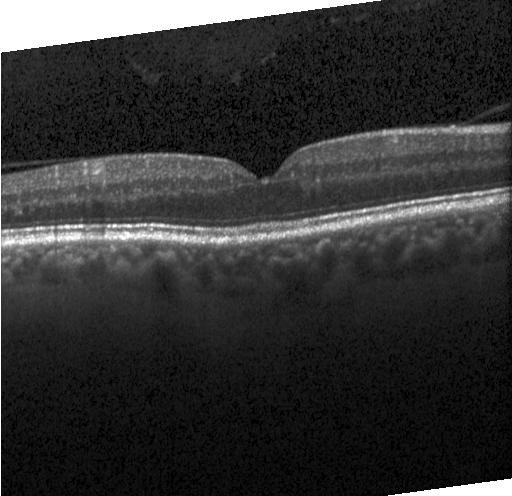

Optical coherence tomography scan, spectral-domain optical coherence tomography. Macular OCT: no choroidal neovascularization, diabetic macular edema, or drusen.